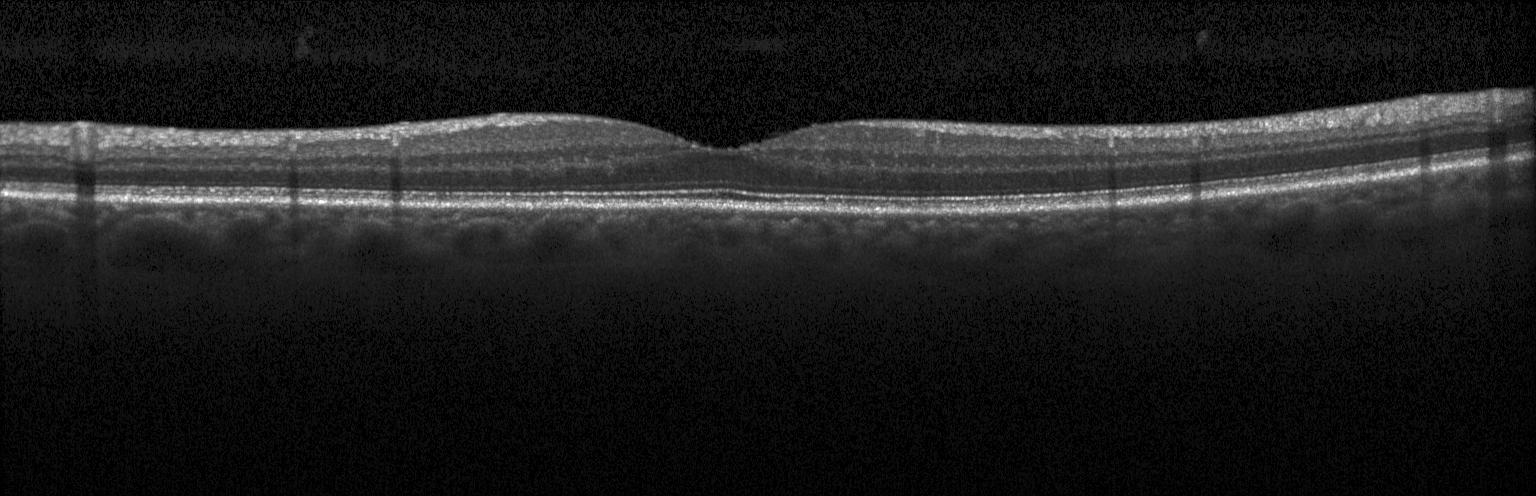 SD-OCT, Heidelberg Spectralis OCT system, retinal OCT B-scan, macular scan.
Impression: no choroidal neovascularization, diabetic macular edema, or drusen.